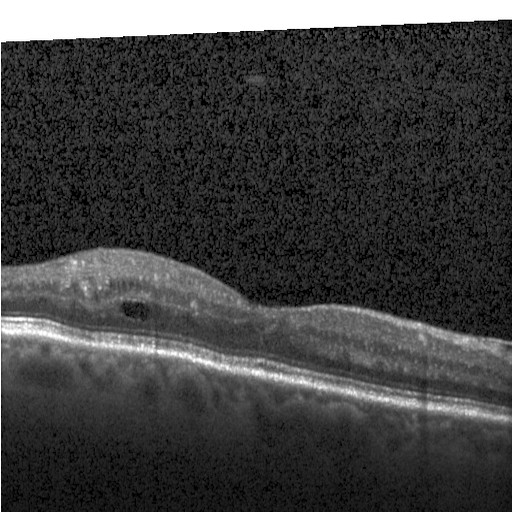
SD-OCT, Heidelberg Spectralis OCT system, OCT B-scan. Finding: diabetic macular edema.